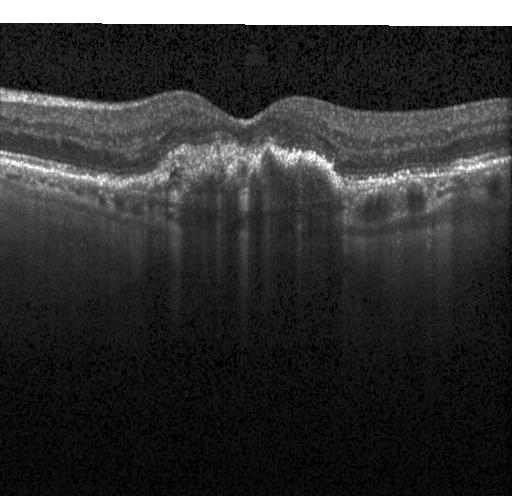 OCT B-scan showing a choroidal neovascular membrane.